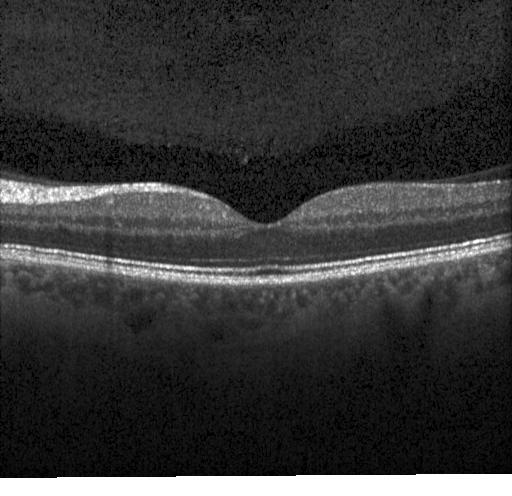
The scan shows no CNV, DME, or drusen.